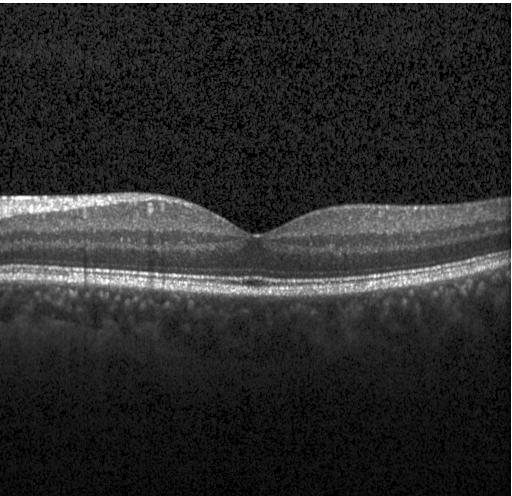

Instrument: Heidelberg Spectralis, horizontal scan through the fovea, optical coherence tomography scan. Macular OCT: no choroidal neovascularization, no diabetic macular edema, and no drusen.